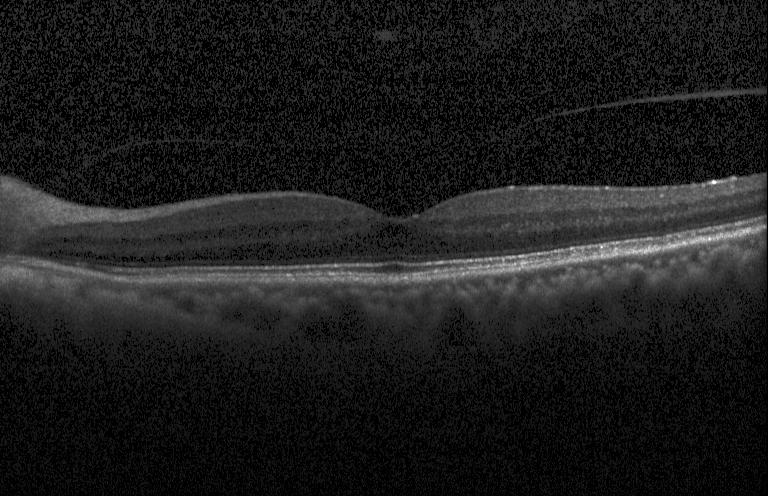 Impression: no evidence of choroidal neovascularization, diabetic macular edema, or drusen.